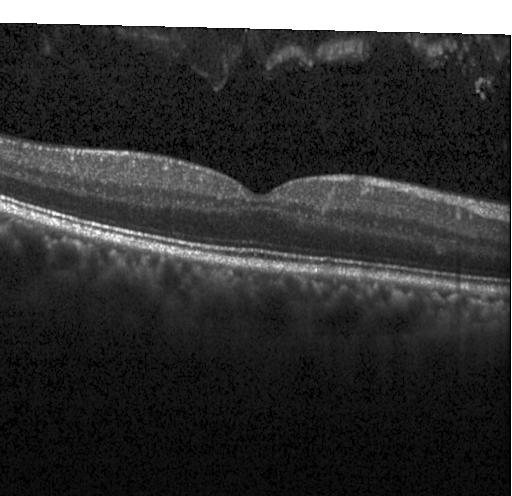 Optical coherence tomography B-scan. Spectral-domain OCT. Centered on the fovea. Heidelberg Spectralis OCT system.
Impression: neither choroidal neovascularization, diabetic macular edema, nor drusen.